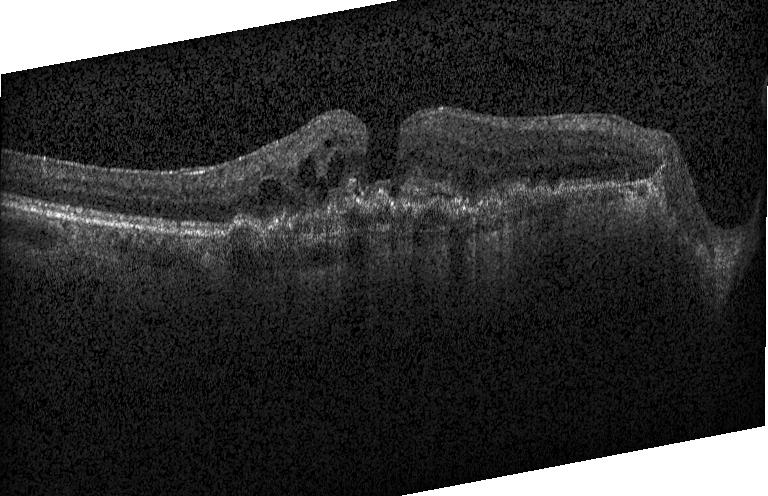
SD-OCT, retinal OCT cross-section, horizontal scan through the fovea, acquired on a Heidelberg Spectralis — Diagnosis: choroidal neovascularization (CNV).